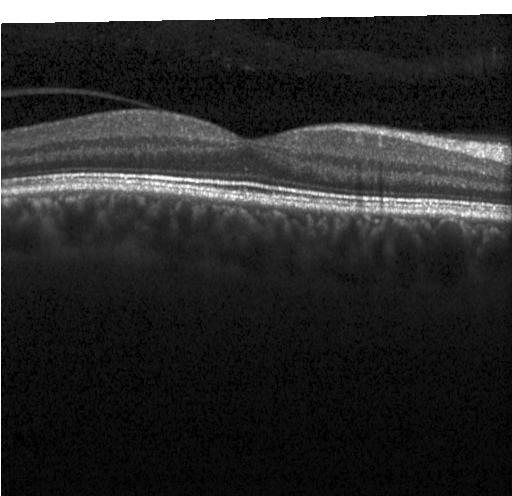

Macular scan, Heidelberg Spectralis, retinal OCT cross-section — The scan shows no evidence of CNV, DME, or drusen.